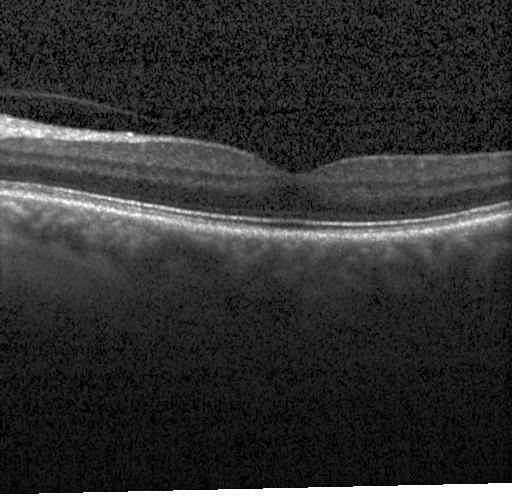

Assessment: no evidence of choroidal neovascularization, diabetic macular edema, or drusen.